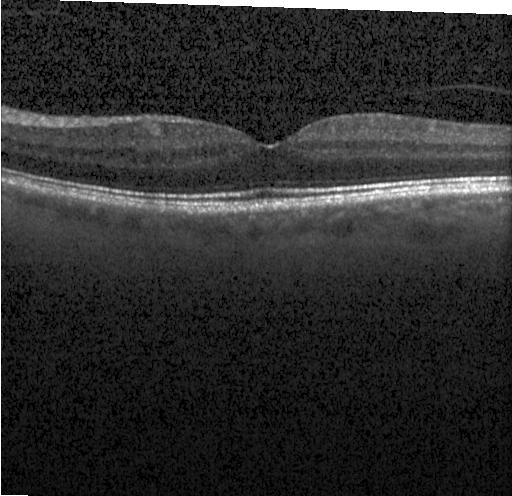 Retinal OCT cross-section.
This B-scan demonstrates no choroidal neovascularization, diabetic macular edema, or drusen.